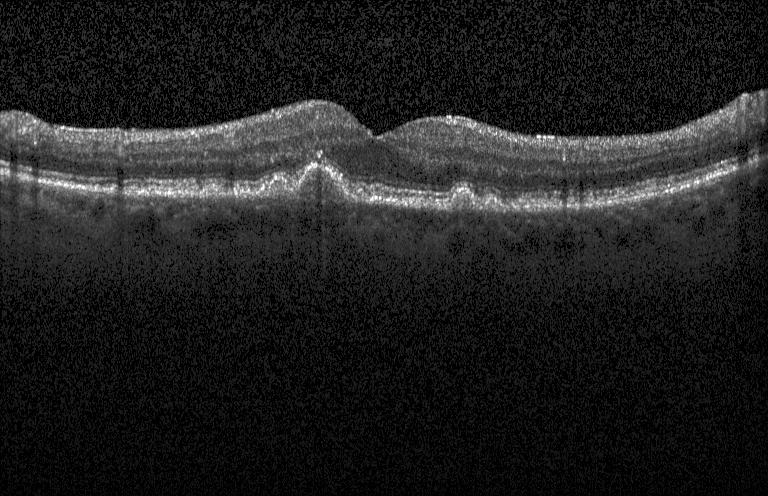 Spectral-domain OCT; instrument: Heidelberg Spectralis; OCT line scan; macular scan.
OCT finding: sub-RPE drusenoid deposits.